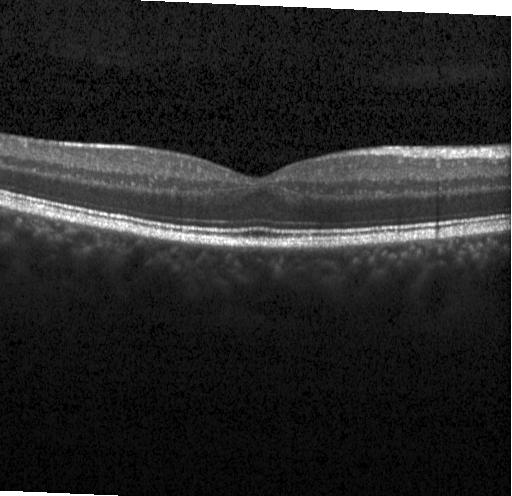

Retinal OCT cross-section — Diagnosis: no choroidal neovascularization, diabetic macular edema, or drusen.